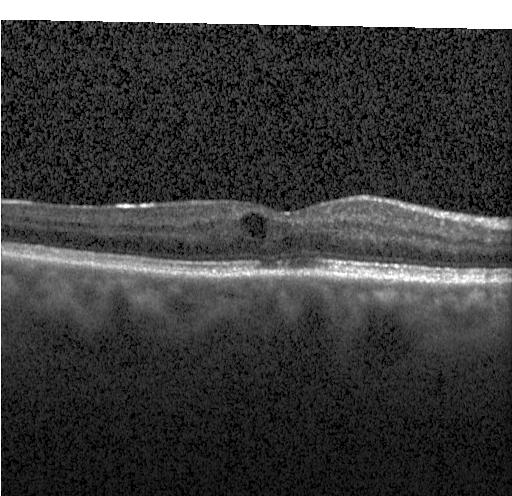
Impression: DME.